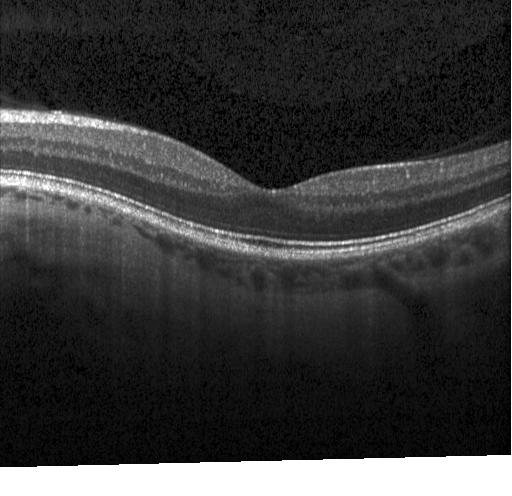 This B-scan demonstrates no evidence of choroidal neovascularization, diabetic macular edema, or drusen.